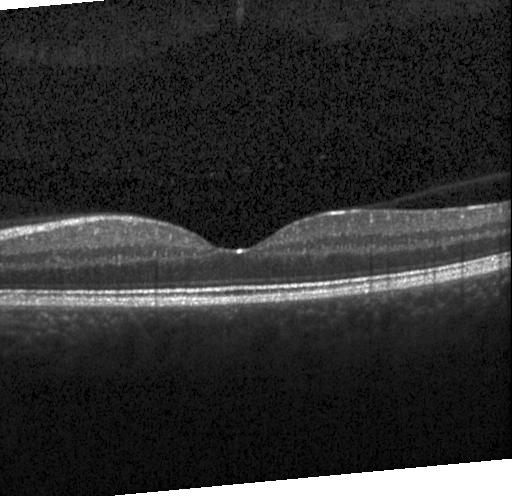 Assessment: no choroidal neovascularization, diabetic macular edema, or drusen.